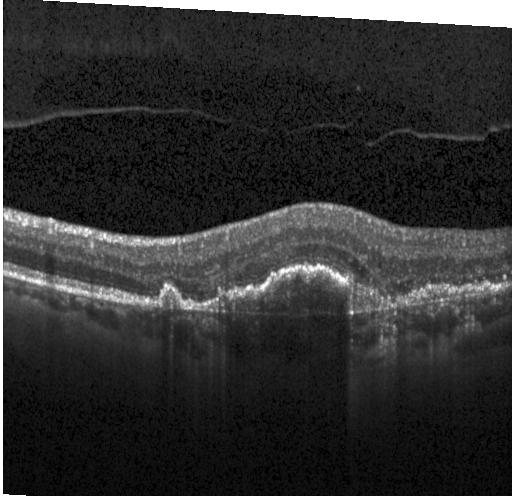
Impression: choroidal neovascularization.